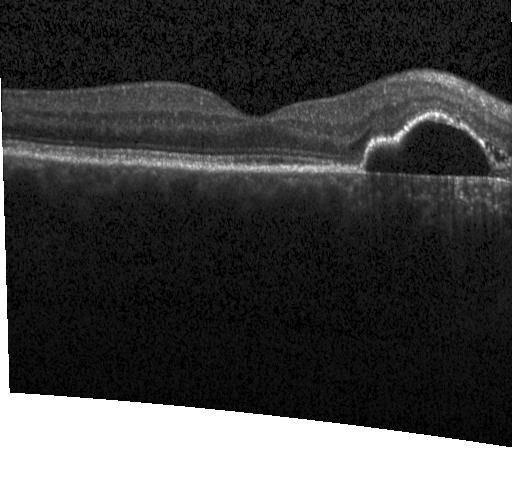
SD-OCT, horizontal scan through the fovea, optical coherence tomography scan. OCT finding: choroidal neovascularization (CNV).